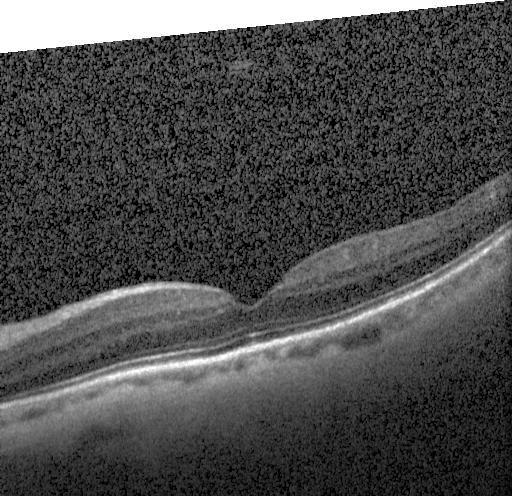
Optical coherence tomography B-scan.
Diagnosis: no choroidal neovascularization, no diabetic macular edema, and no drusen.